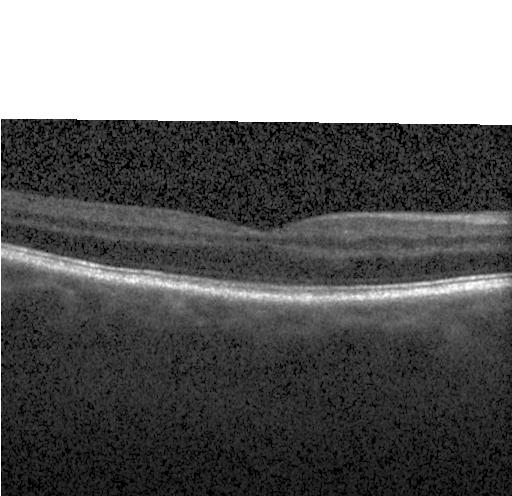
OCT scan showing no choroidal neovascularization, no diabetic macular edema, and no drusen.